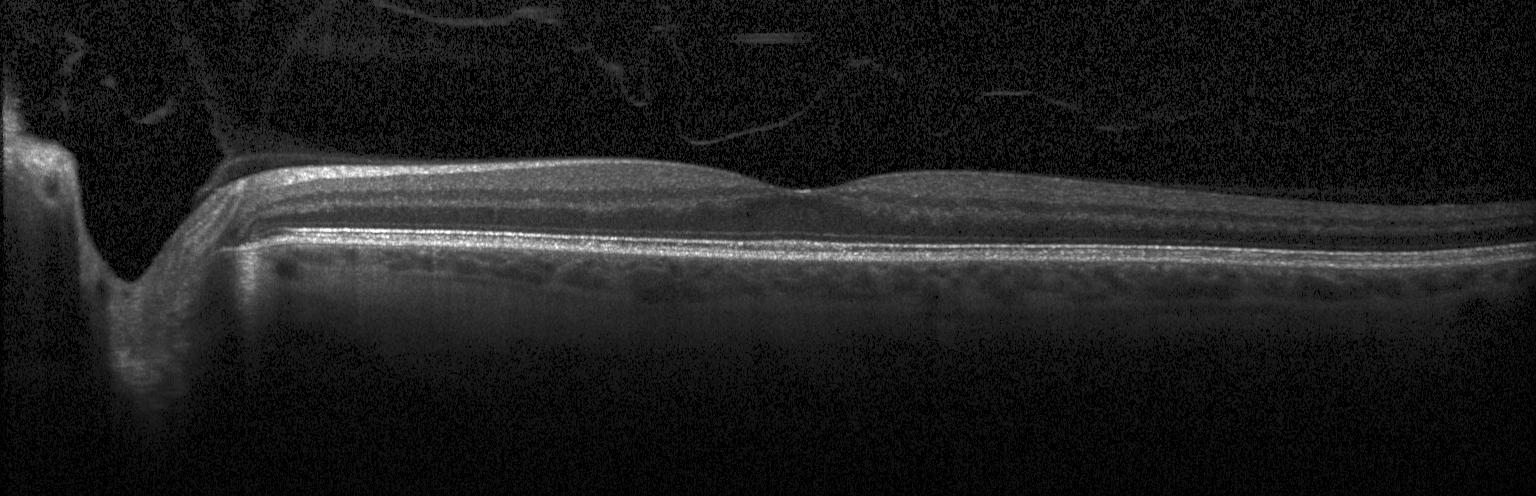

This B-scan demonstrates no CNV, DME, or drusen.